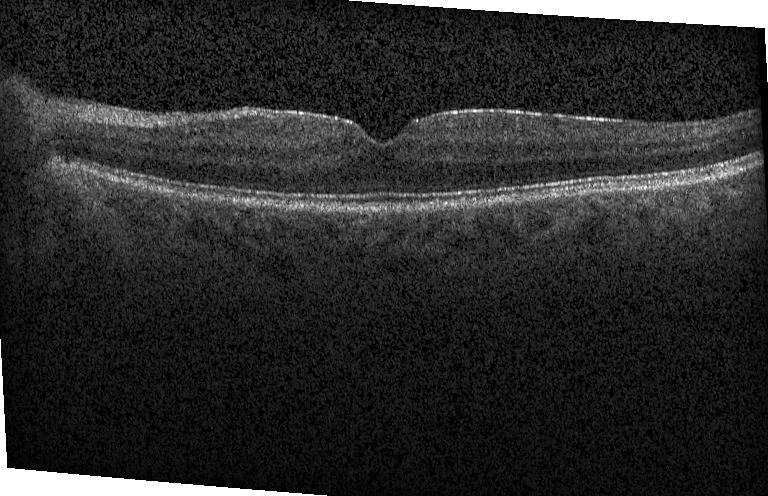
The scan shows neither choroidal neovascularization, diabetic macular edema, nor drusen.